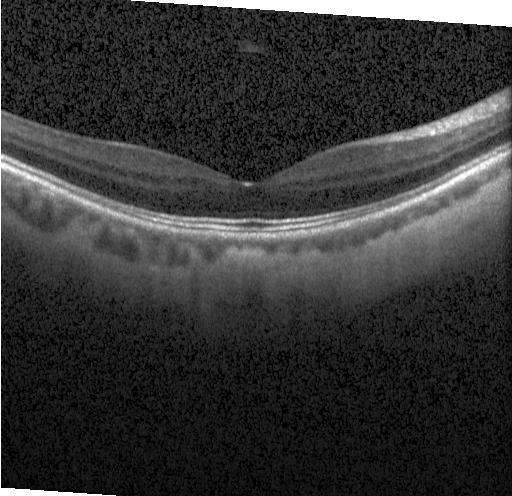

No choroidal neovascularization, diabetic macular edema, or drusen.